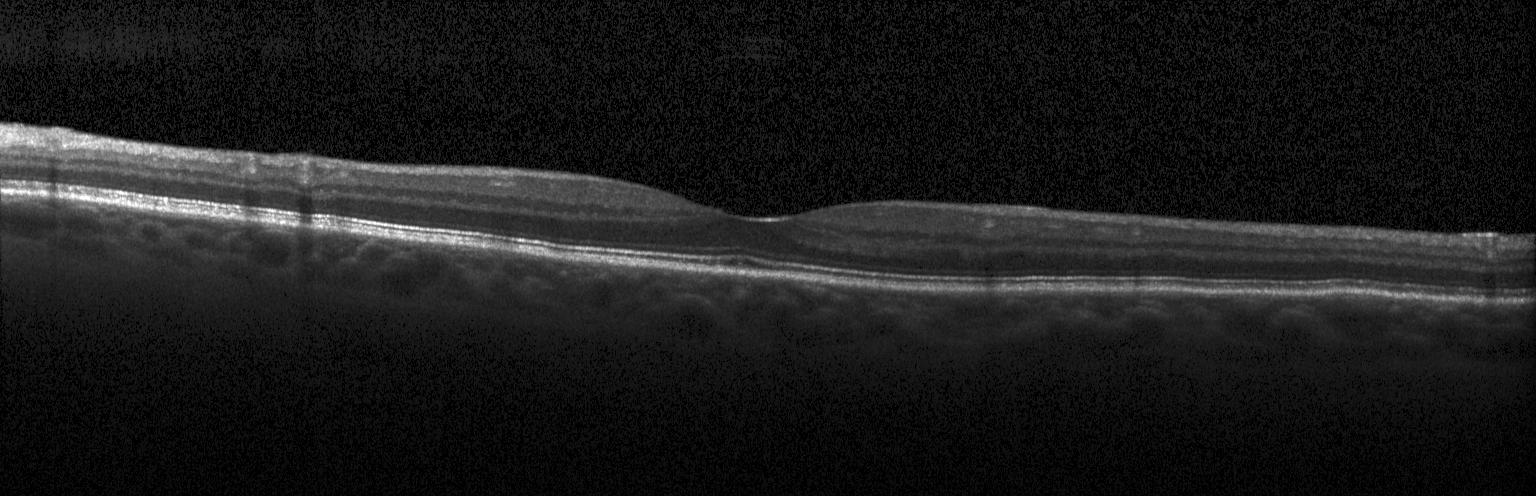
OCT line scan; spectral-domain OCT — Impression: neither CNV, DME, nor drusen.